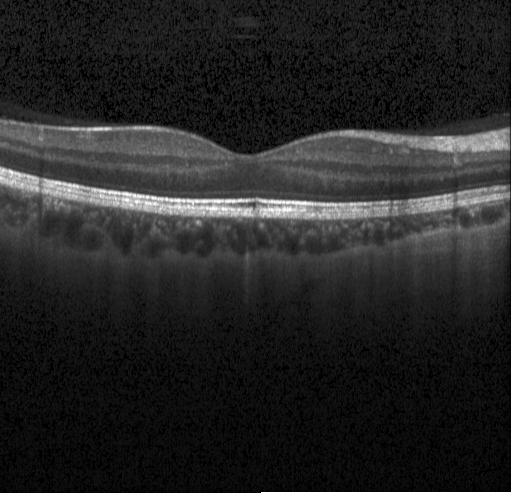 Assessment: neither choroidal neovascularization, diabetic macular edema, nor drusen.